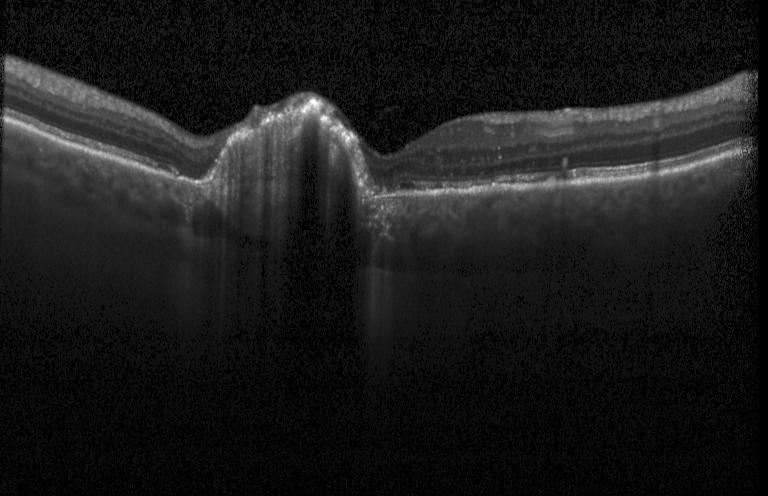

Spectral-domain optical coherence tomography, optical coherence tomography scan, instrument: Heidelberg Spectralis — Assessment: a choroidal neovascular membrane.